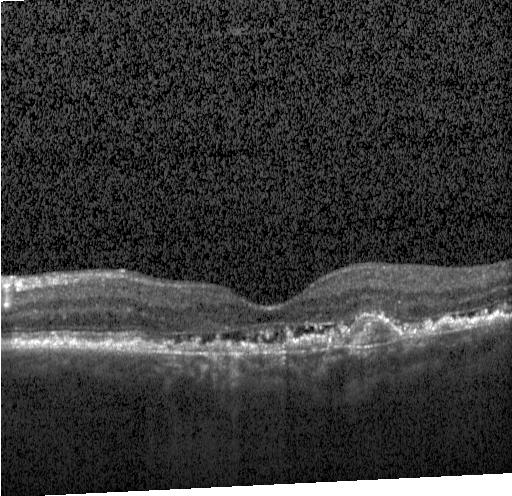
Macular scan. Retinal OCT B-scan.
Diagnosis: a choroidal neovascular membrane.